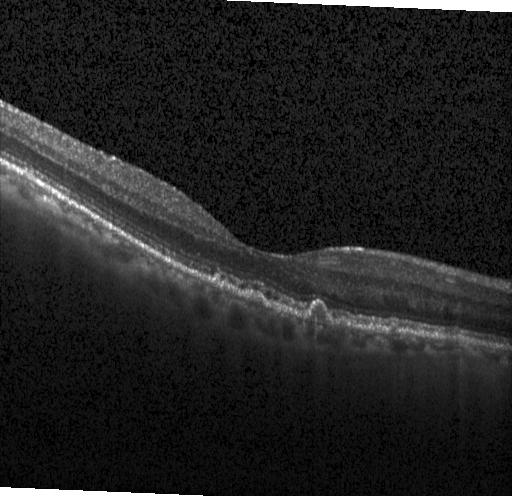 Retinal OCT cross-section — The scan shows drusen.